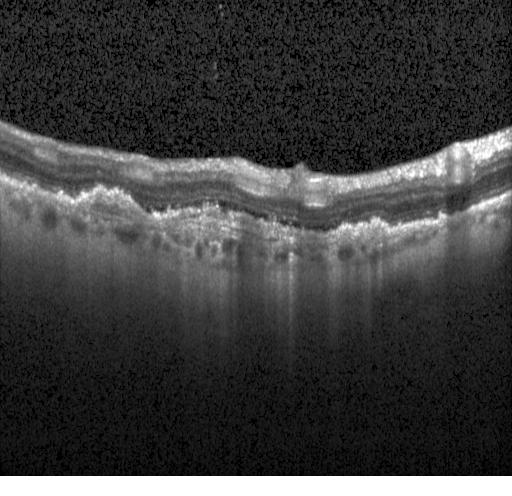

A choroidal neovascular membrane.